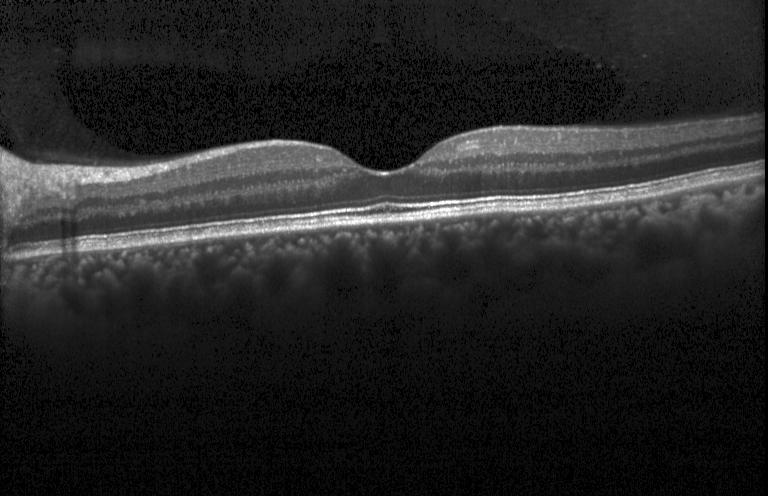
Macular scan · retinal OCT B-scan · instrument: Heidelberg Spectralis
Impression: no choroidal neovascularization, diabetic macular edema, or drusen.